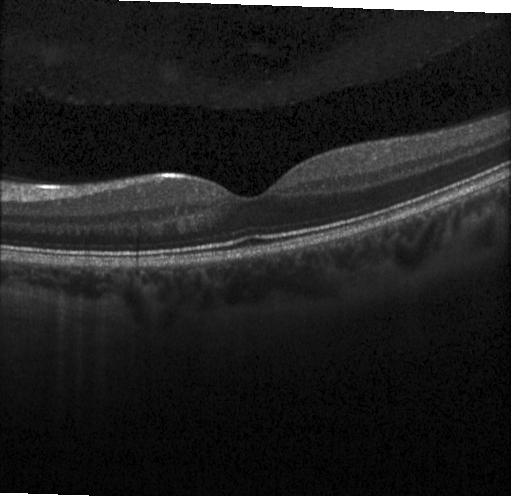 Macular OCT demonstrating no CNV, no DME, and no drusen.